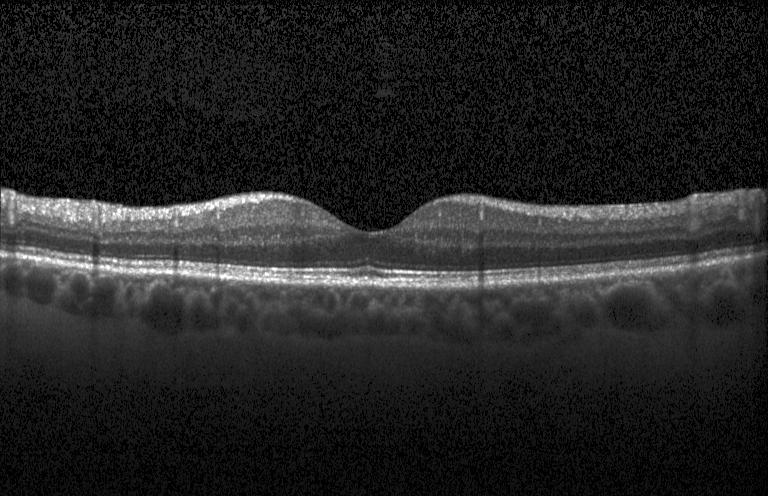

OCT finding: no evidence of choroidal neovascularization, diabetic macular edema, or drusen.